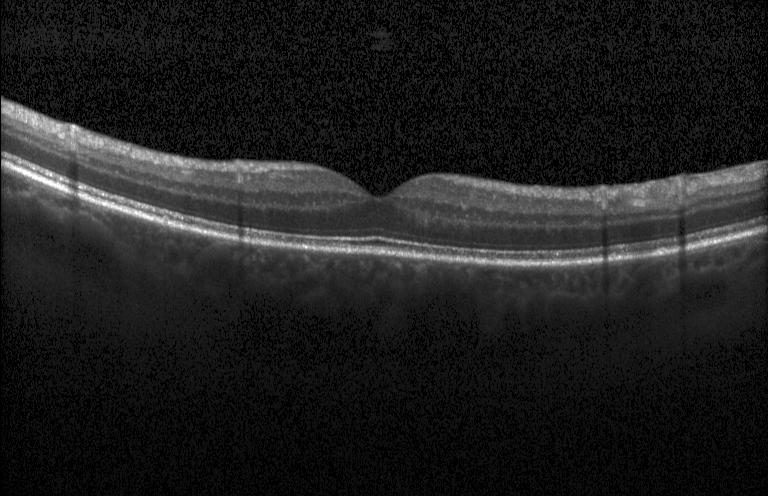
Heidelberg Spectralis OCT system · OCT line scan · horizontal scan through the fovea · spectral-domain optical coherence tomography — This B-scan demonstrates no choroidal neovascularization, diabetic macular edema, or drusen.